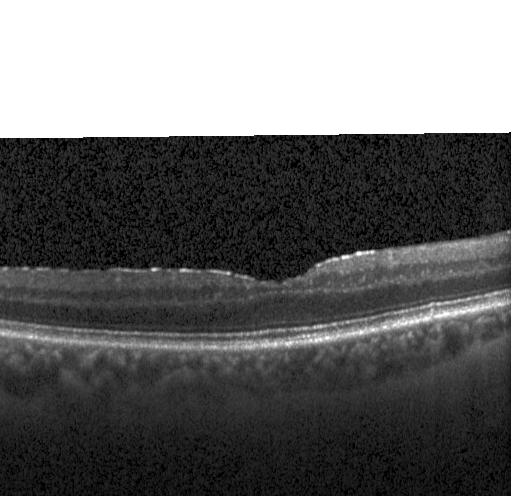

OCT B-scan · spectral-domain OCT. No evidence of CNV, DME, or drusen.